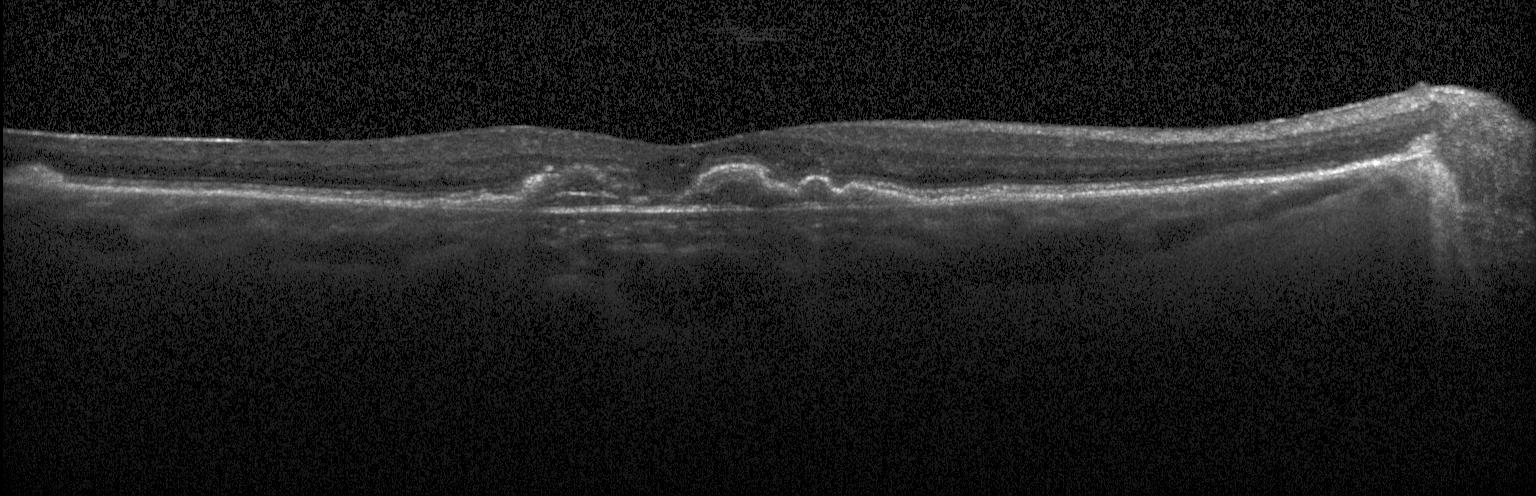

Retinal OCT B-scan, instrument: Heidelberg Spectralis
Assessment: a choroidal neovascular membrane.